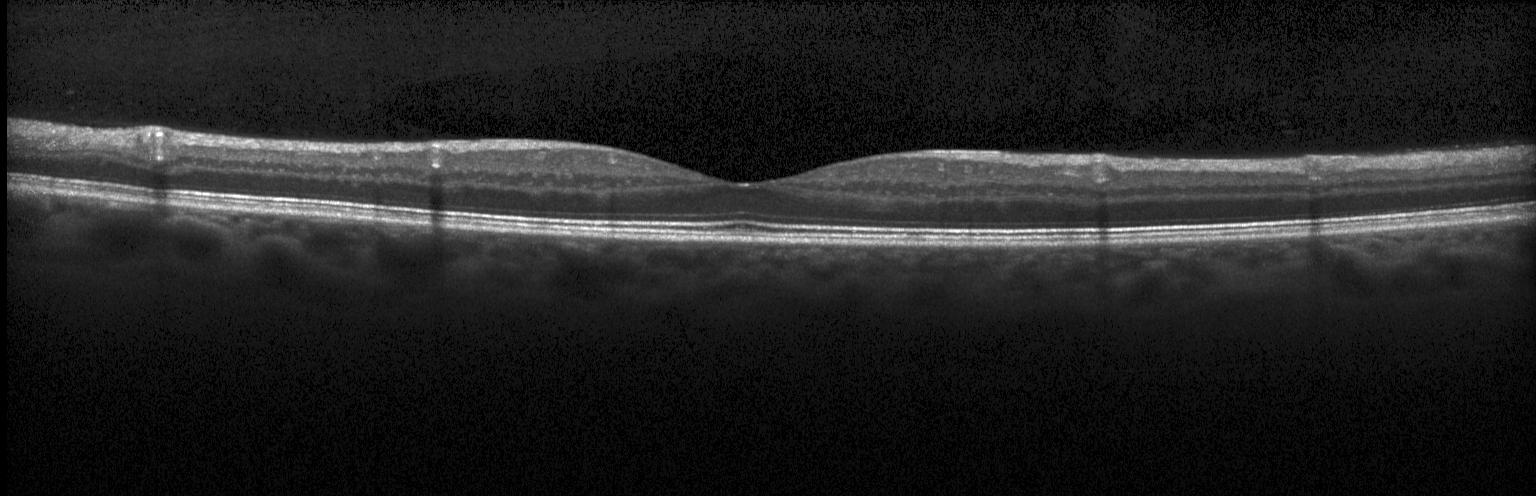

Impression: no choroidal neovascularization, diabetic macular edema, or drusen.